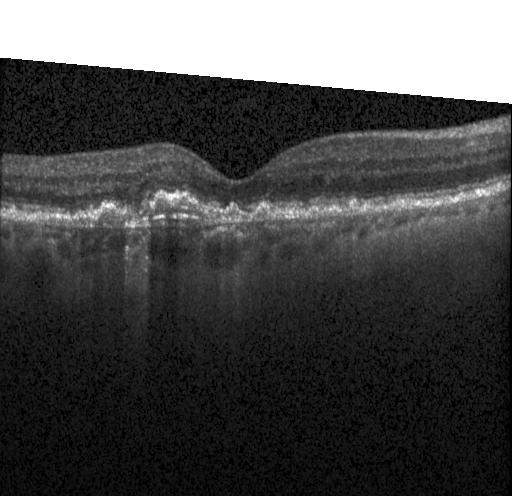
Assessment: choroidal neovascularization.